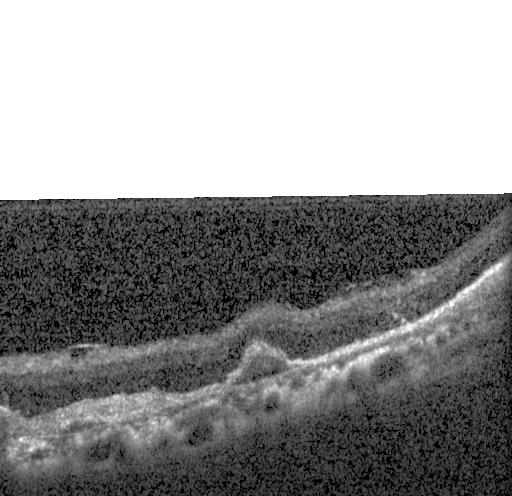
Impression: a choroidal neovascular membrane.